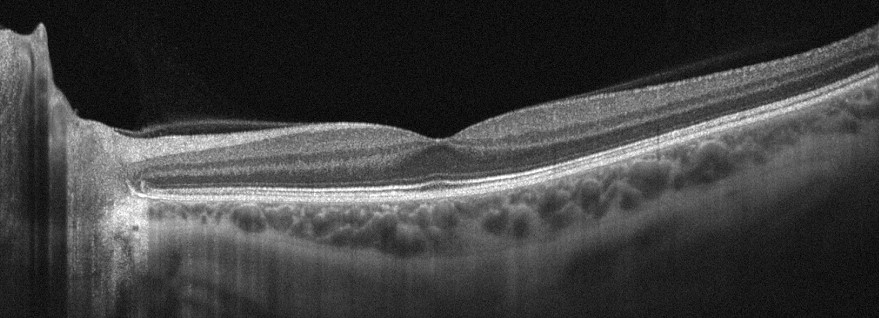

Macular OCT: absence of AMD, DME, ERM, RAO, RVO, and vitreomacular interface disease.